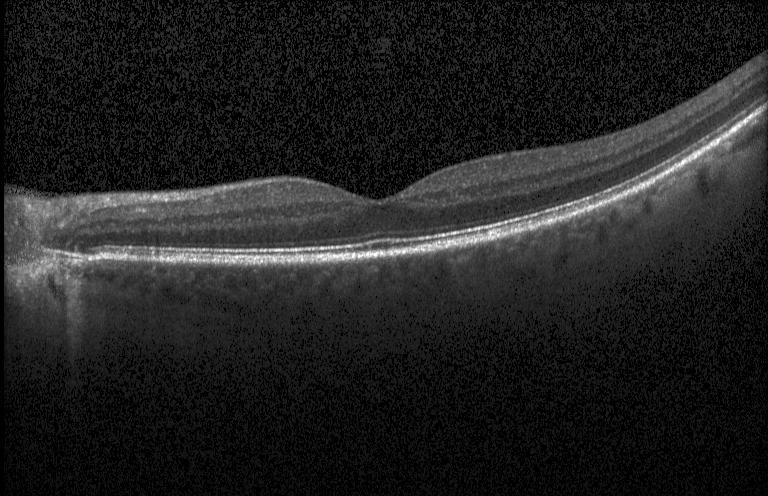

Fovea-centered; instrument: Heidelberg Spectralis; SD-OCT; optical coherence tomography B-scan.
Finding: no CNV, DME, or drusen.